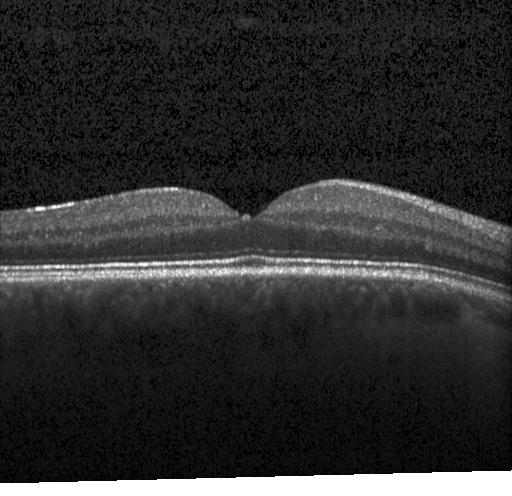 OCT B-scan — Macular OCT: no choroidal neovascularization, no diabetic macular edema, and no drusen.